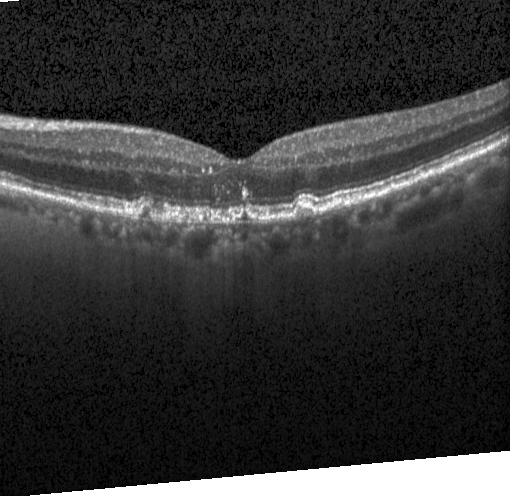 Retinal OCT cross-section.
Finding: drusen.